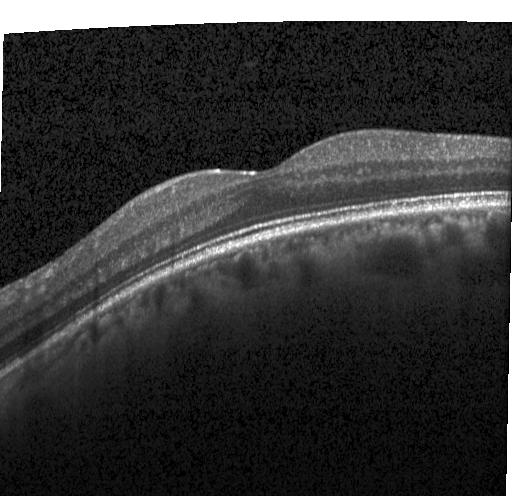

Spectral-domain OCT, Heidelberg Spectralis, macular scan, optical coherence tomography B-scan.
OCT finding: neither choroidal neovascularization, diabetic macular edema, nor drusen.